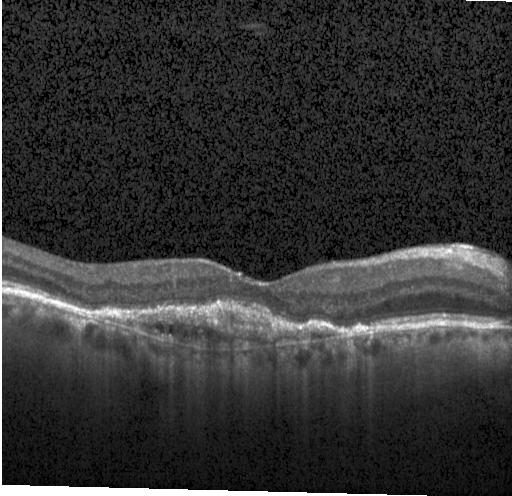
OCT line scan.
OCT finding: choroidal neovascularization.